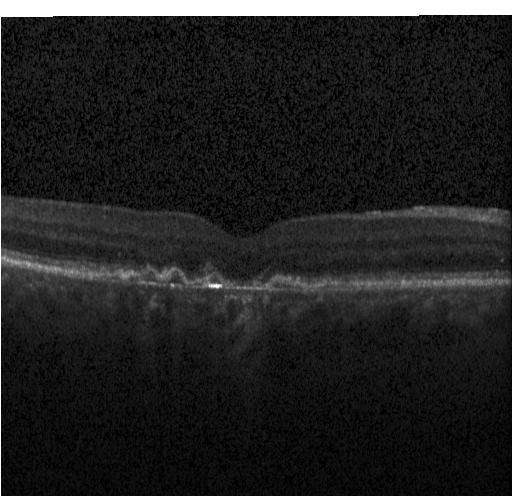

Impression: CNV.